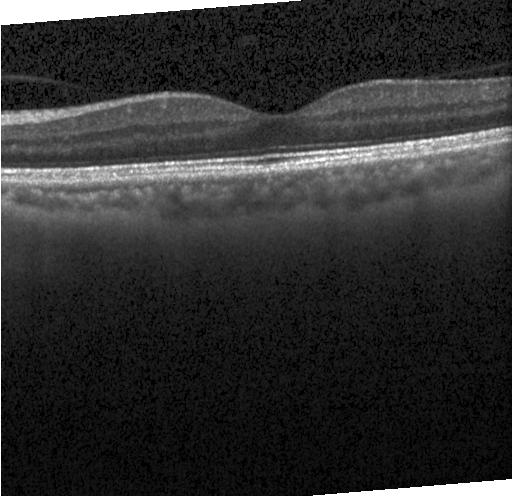
Macular scan; spectral-domain OCT; Heidelberg Spectralis OCT system; retinal OCT B-scan. Diagnosis: neither choroidal neovascularization, diabetic macular edema, nor drusen.